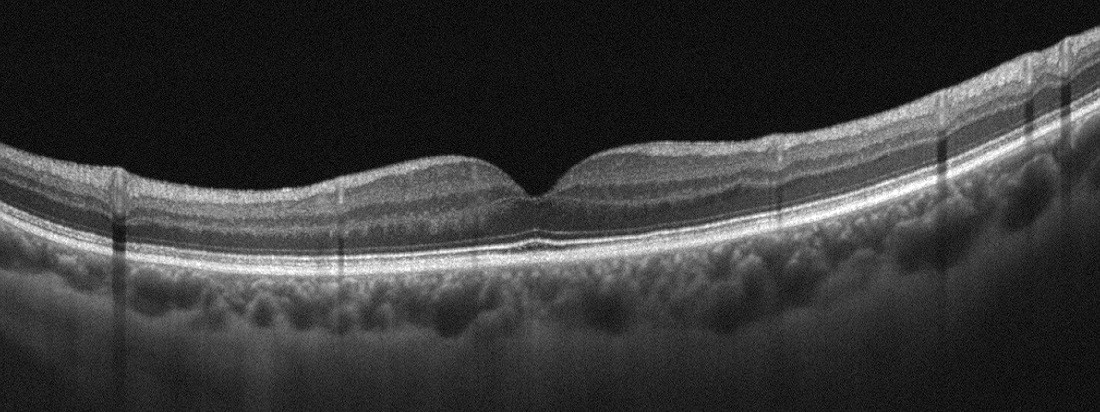 Macular OCT demonstrating absence of AMD, DME, ERM, RAO, RVO, and vitreomacular interface disease.